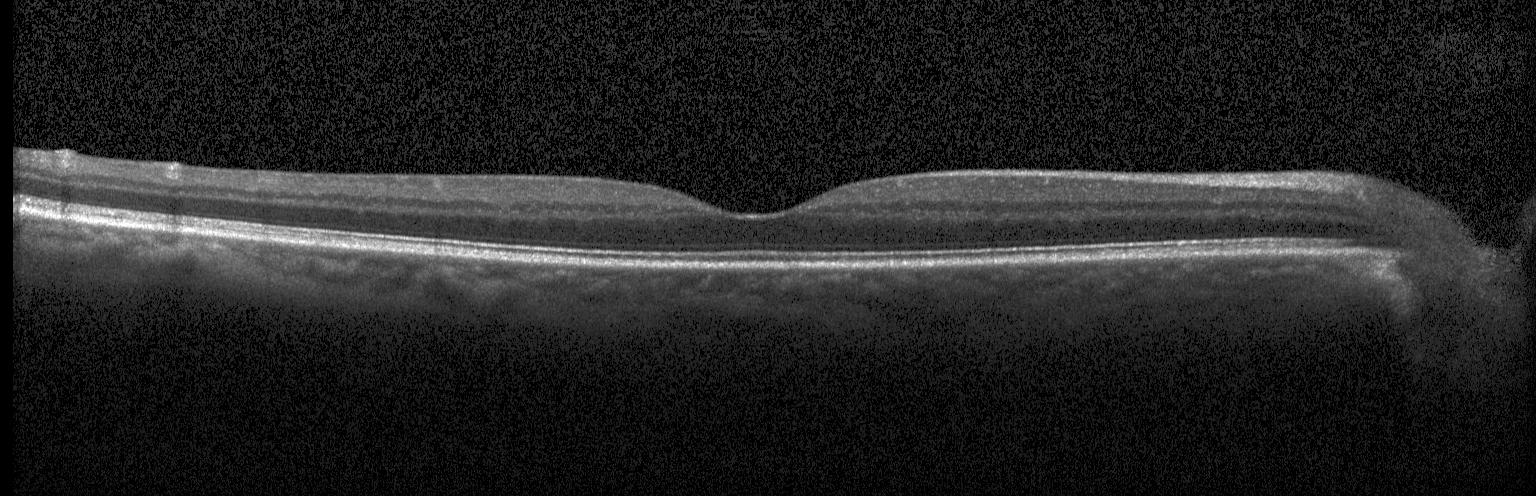

Retinal OCT B-scan · instrument: Heidelberg Spectralis
Macular OCT: no choroidal neovascularization, diabetic macular edema, or drusen.